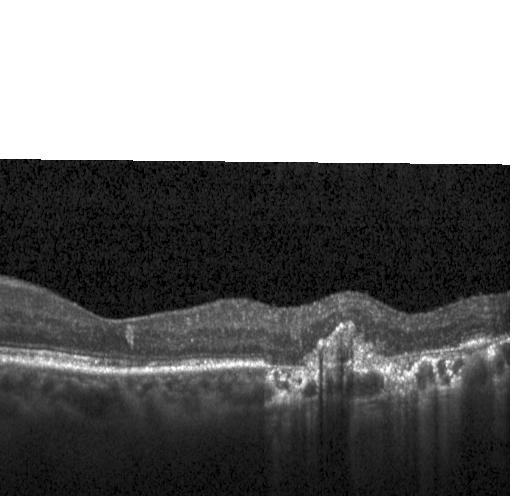

Retinal OCT cross-section.
Assessment: CNV.